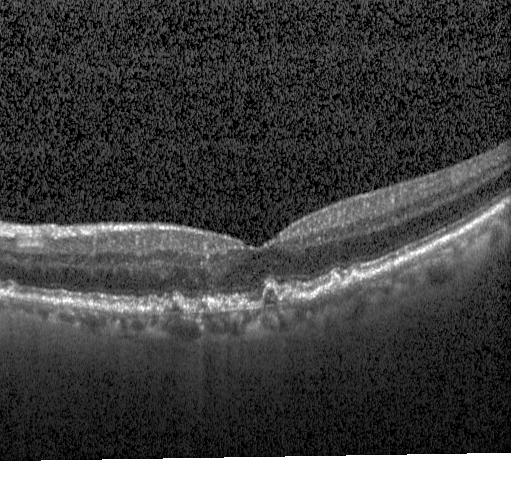

Optical coherence tomography scan. Heidelberg Spectralis. SD-OCT. Horizontal scan through the fovea.
This B-scan demonstrates choroidal neovascularization.